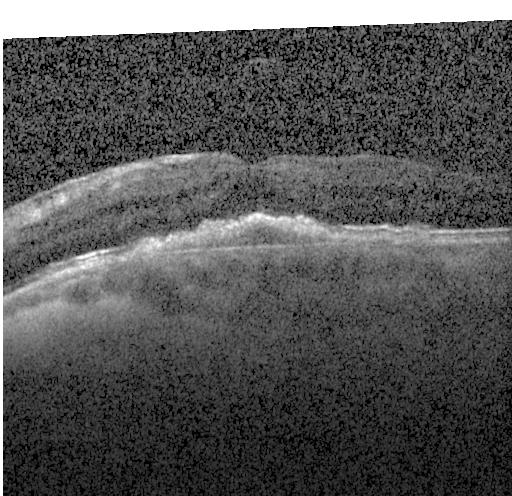
Macular OCT: choroidal neovascularization (CNV).